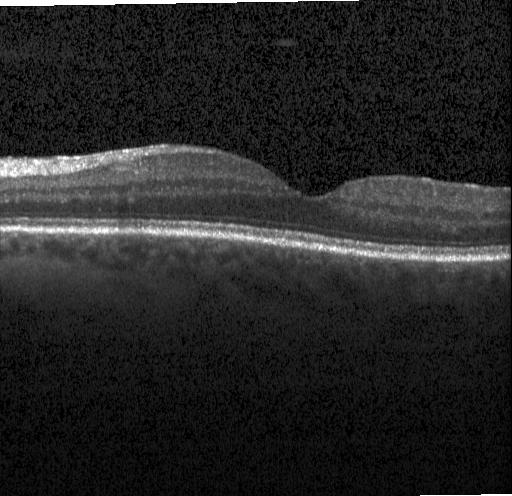
Horizontal scan through the fovea; optical coherence tomography scan. Impression: no choroidal neovascularization, no diabetic macular edema, and no drusen.